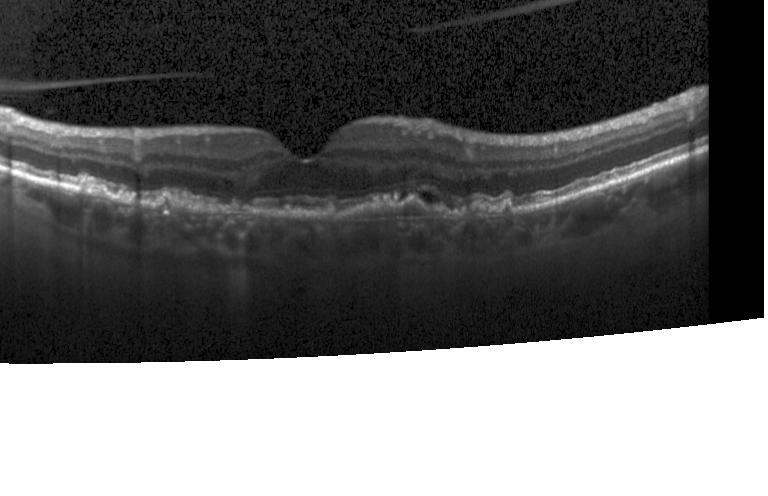
Retinal OCT cross-section showing a choroidal neovascular membrane.